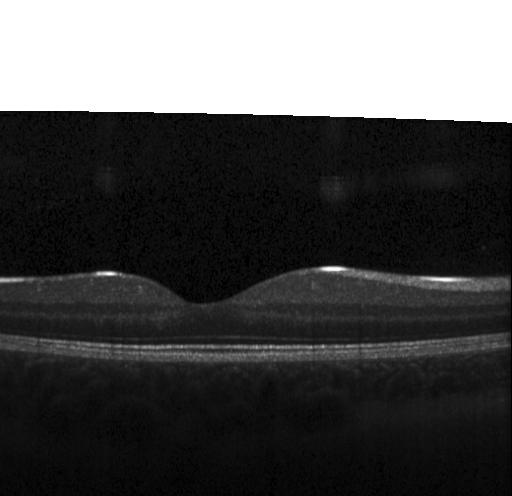 Heidelberg Spectralis OCT system · optical coherence tomography scan · SD-OCT · through the macula — Dx: no choroidal neovascularization, no diabetic macular edema, and no drusen.